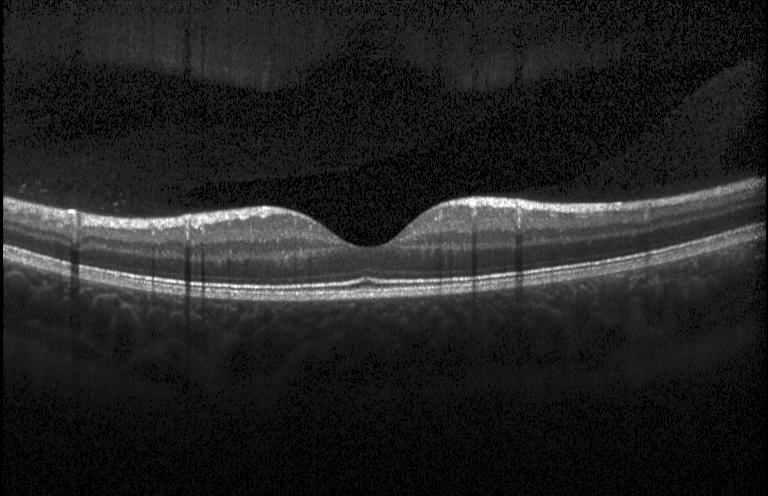 OCT line scan.
OCT finding: no choroidal neovascularization, diabetic macular edema, or drusen.